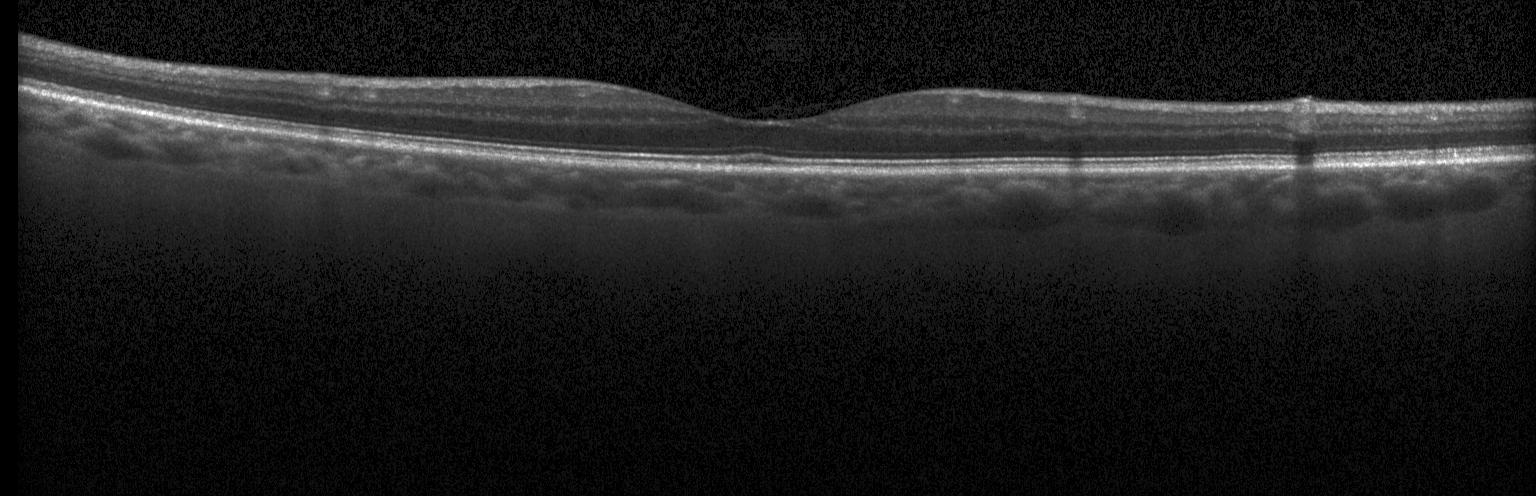
Finding: no choroidal neovascularization, no diabetic macular edema, and no drusen.